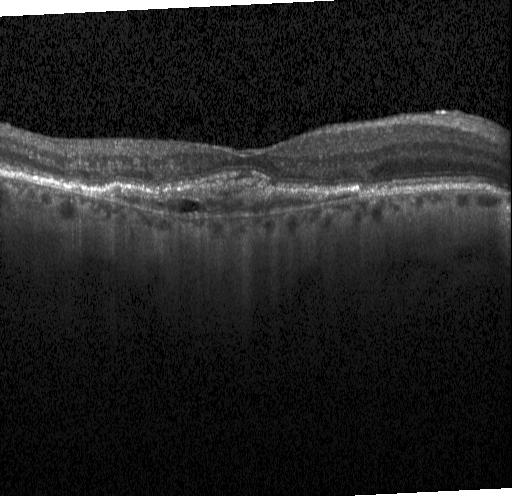
Spectral-domain optical coherence tomography · retinal OCT cross-section — A choroidal neovascular membrane.